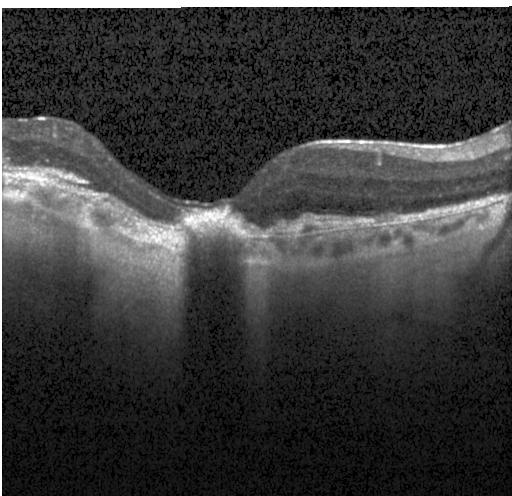

OCT line scan.
Macular OCT: a choroidal neovascular membrane.